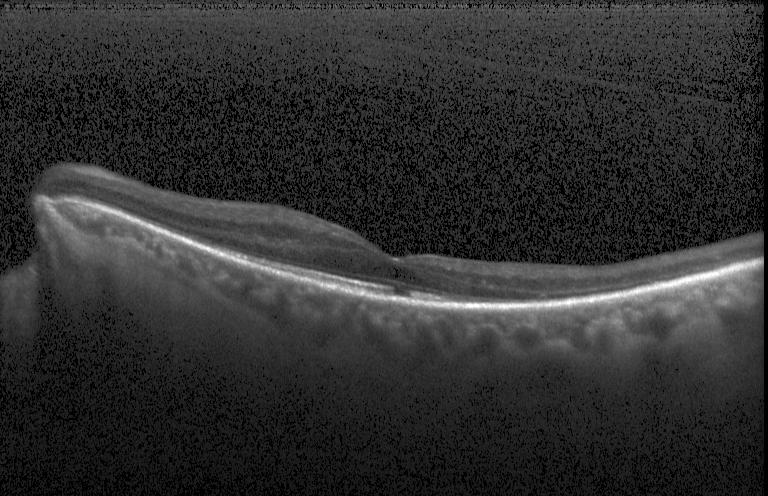

Finding: no evidence of choroidal neovascularization, diabetic macular edema, or drusen.